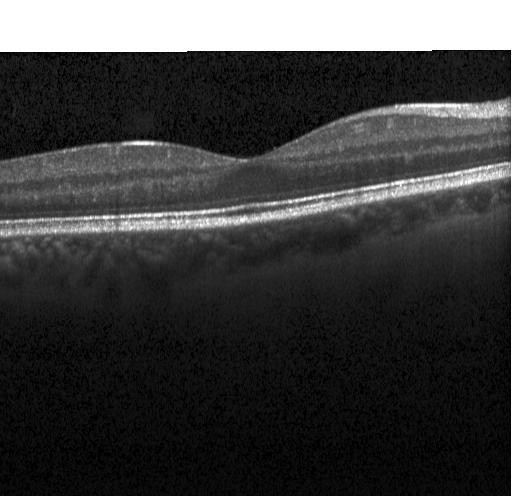

Optical coherence tomography scan.
Assessment: no CNV, DME, or drusen.